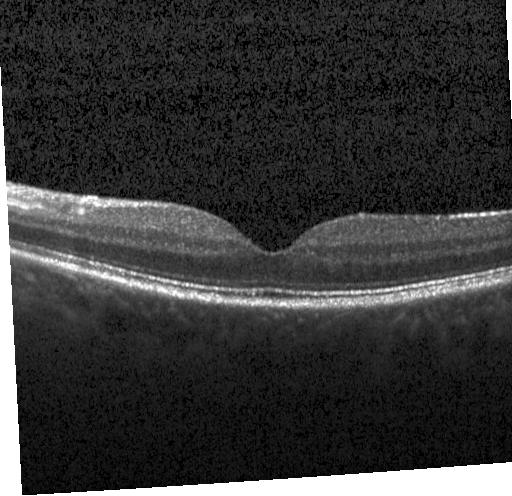
Assessment: neither CNV, DME, nor drusen.